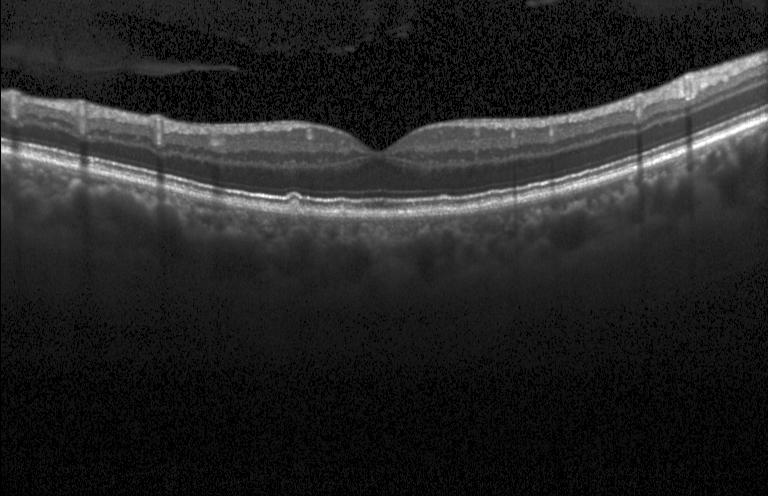
Retinal OCT B-scan. Spectral-domain optical coherence tomography
Diagnosis: drusen.